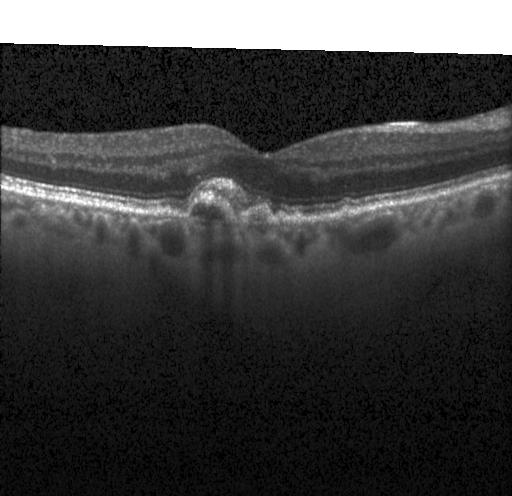
Assessment: a choroidal neovascular membrane.